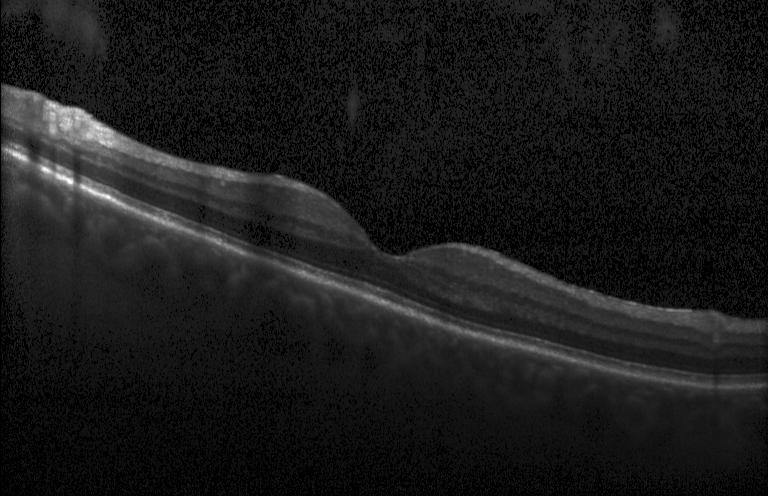

Macular OCT demonstrating no evidence of choroidal neovascularization, diabetic macular edema, or drusen.